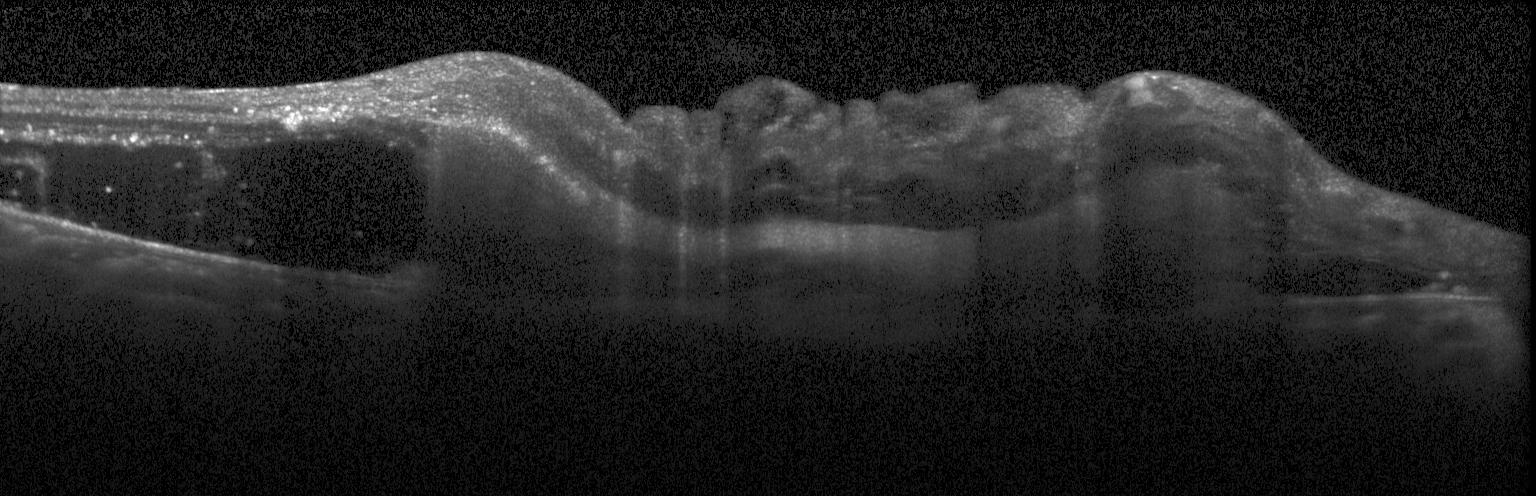

Spectral-domain OCT B-scan: a choroidal neovascular membrane.